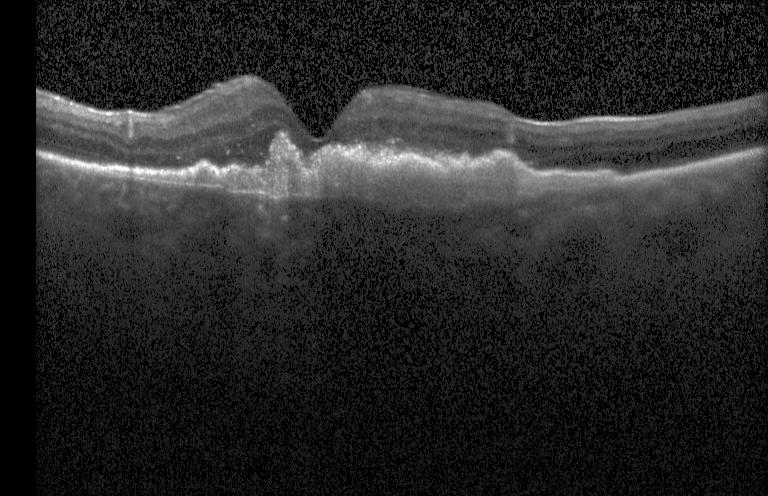 Horizontal scan through the fovea. Optical coherence tomography B-scan. Dx: a choroidal neovascular membrane.